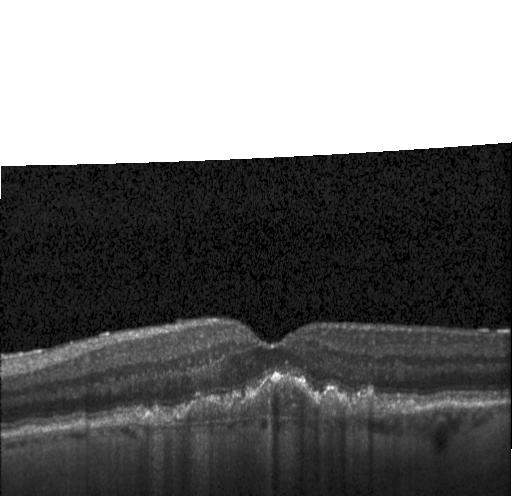

Fovea-centered. Retinal OCT B-scan. Dx: choroidal neovascularization (CNV).